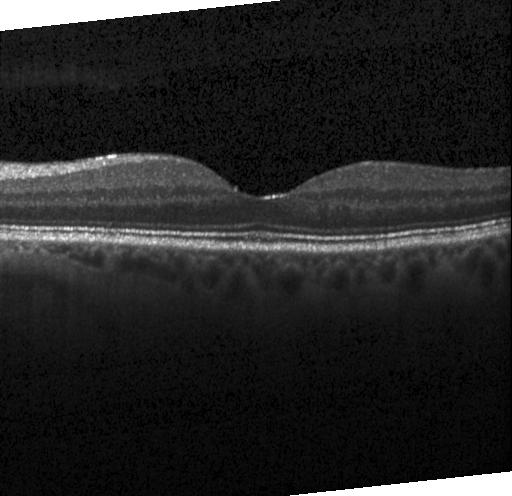

Diagnosis: no evidence of choroidal neovascularization, diabetic macular edema, or drusen.